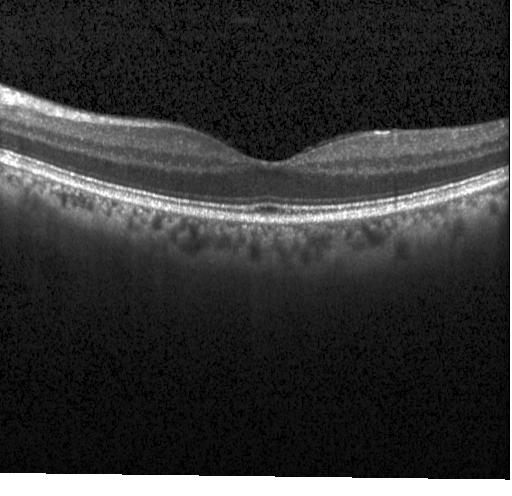
OCT finding: no choroidal neovascularization, diabetic macular edema, or drusen.